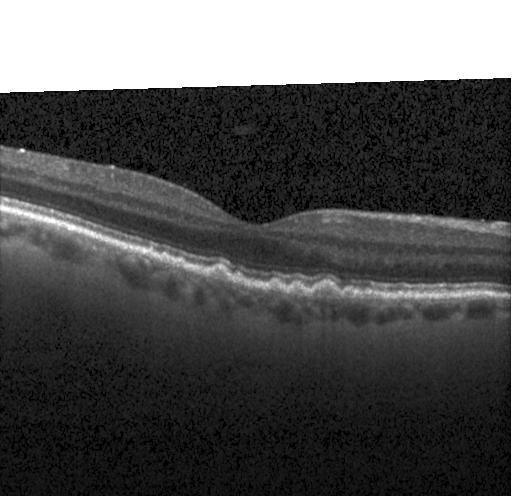
Heidelberg Spectralis OCT system, retinal OCT cross-section.
Impression: sub-RPE drusenoid deposits.